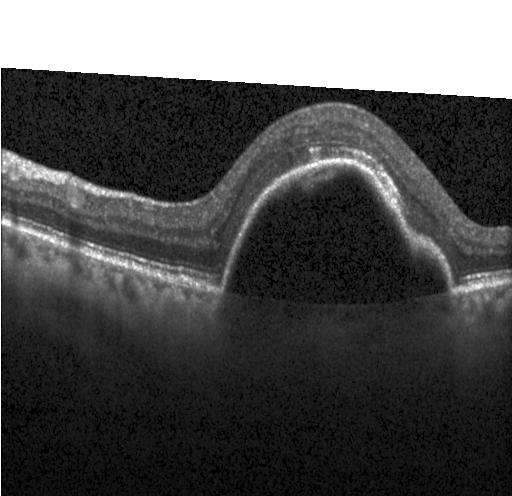 OCT finding: choroidal neovascularization (CNV).